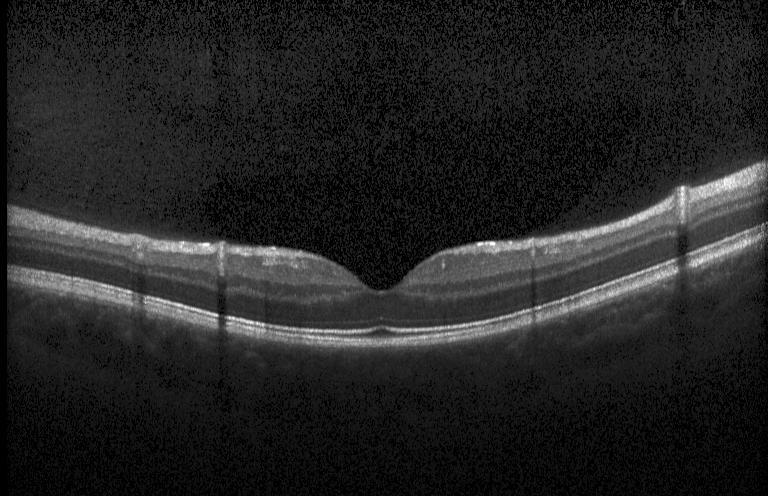

OCT line scan, through the macula, Heidelberg Spectralis, SD-OCT.
Dx: no evidence of choroidal neovascularization, diabetic macular edema, or drusen.